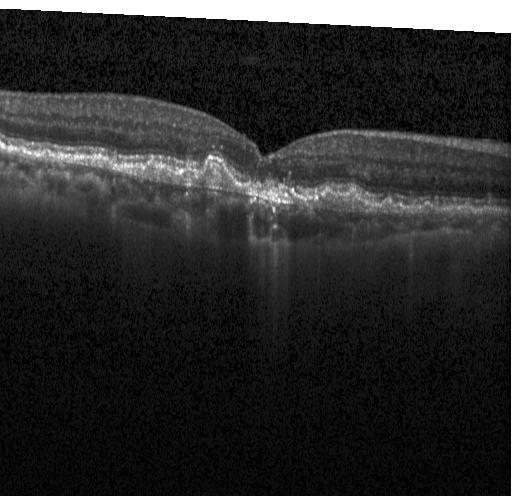

Macular OCT: a choroidal neovascular membrane.